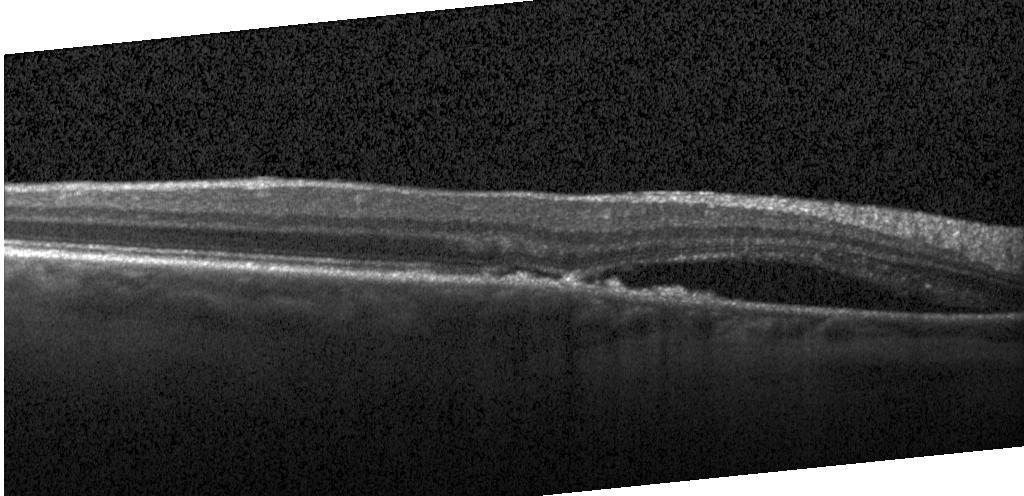
Fovea-centered; acquired on a Heidelberg Spectralis; spectral-domain OCT; optical coherence tomography scan
Choroidal neovascularization (CNV).